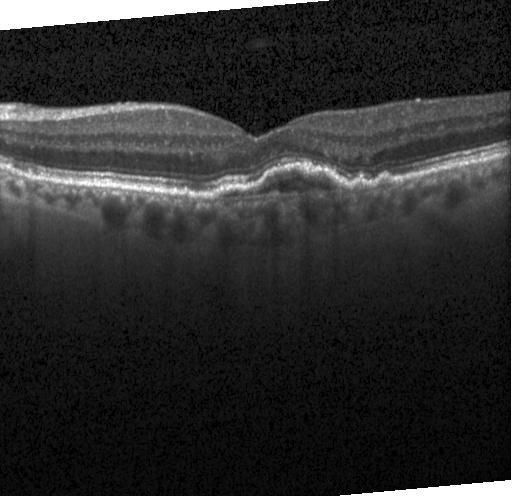

OCT line scan.
This B-scan demonstrates a choroidal neovascular membrane.